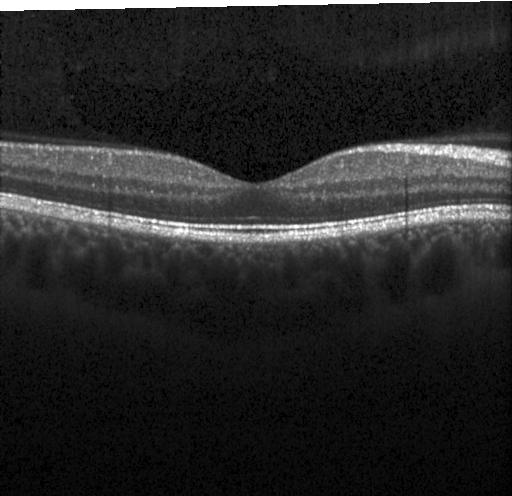
SD-OCT · Heidelberg Spectralis · OCT B-scan · horizontal scan through the fovea.
Assessment: no CNV, DME, or drusen.